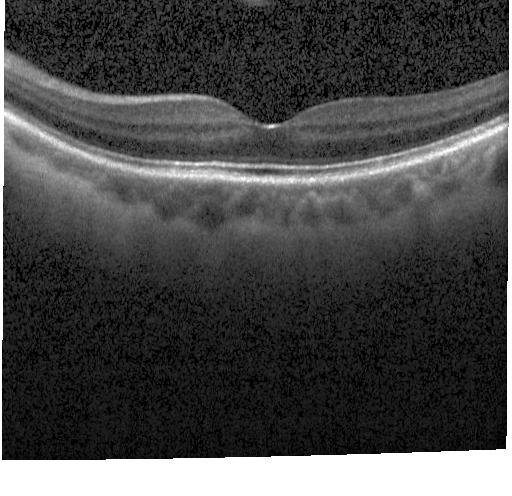

Retinal OCT cross-section · acquired on a Heidelberg Spectralis · SD-OCT. Dx: neither choroidal neovascularization, diabetic macular edema, nor drusen.